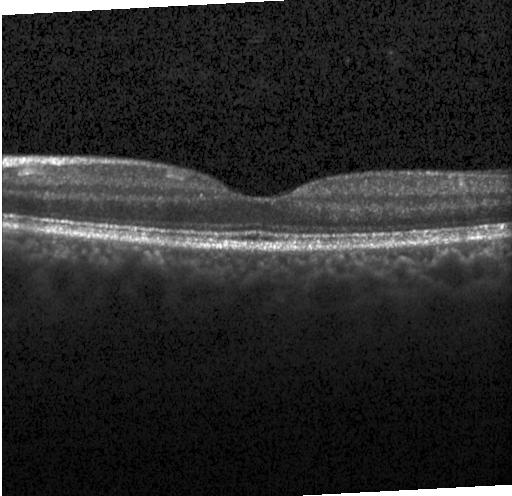

OCT B-scan — Assessment: no choroidal neovascularization, no diabetic macular edema, and no drusen.